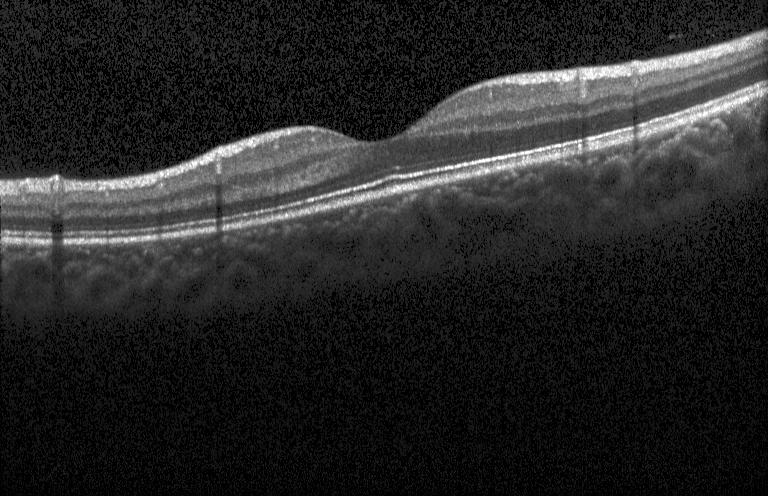

The scan shows neither choroidal neovascularization, diabetic macular edema, nor drusen.